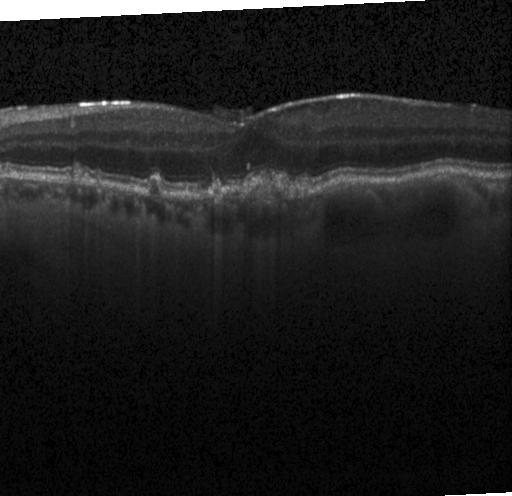
Macular OCT: drusen.